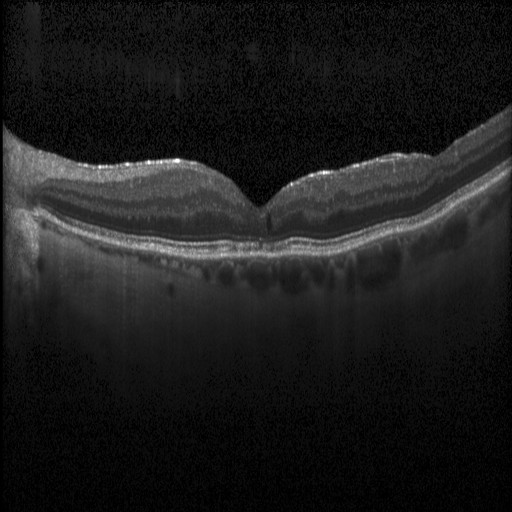 Instrument: Heidelberg Spectralis, optical coherence tomography B-scan.
OCT finding: diabetic macular edema.